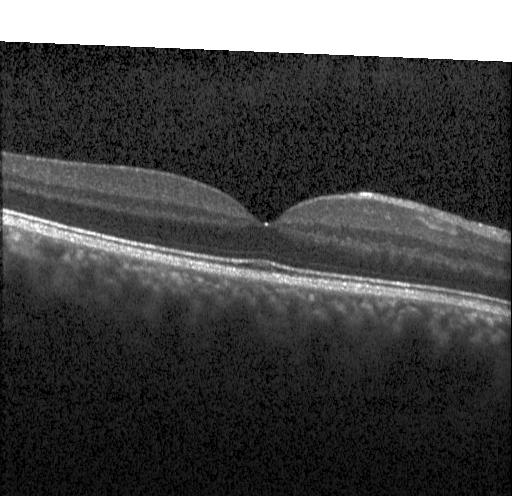
Retinal OCT cross-section
Impression: no CNV, no DME, and no drusen.